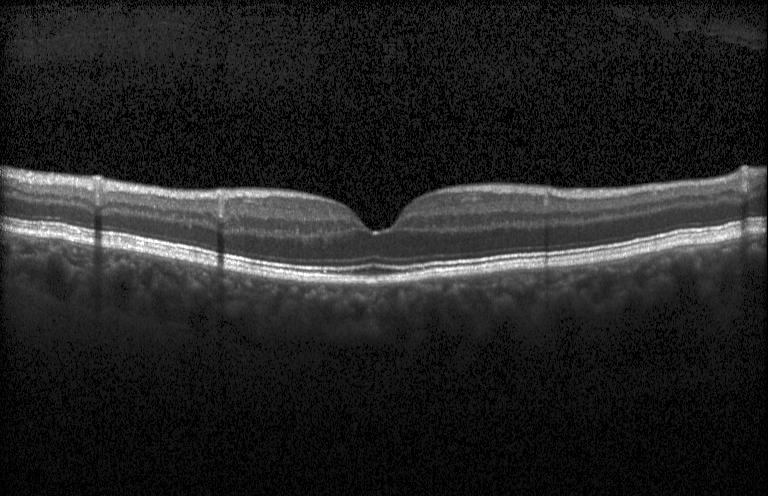
Impression: neither choroidal neovascularization, diabetic macular edema, nor drusen.